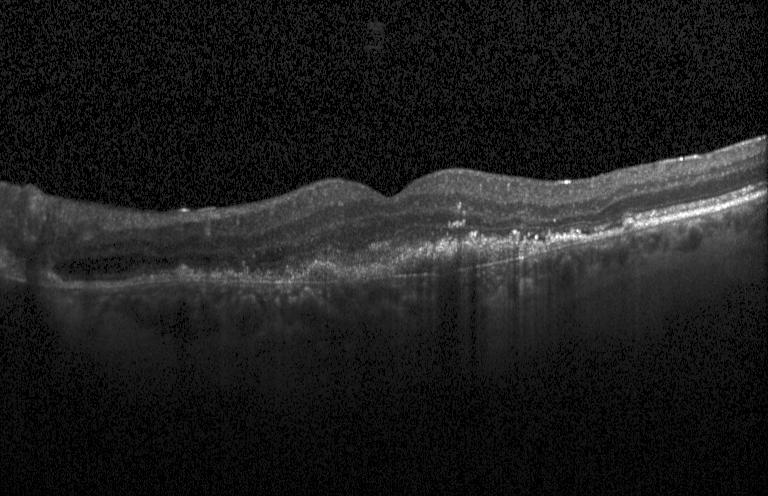
Finding: choroidal neovascularization (CNV).